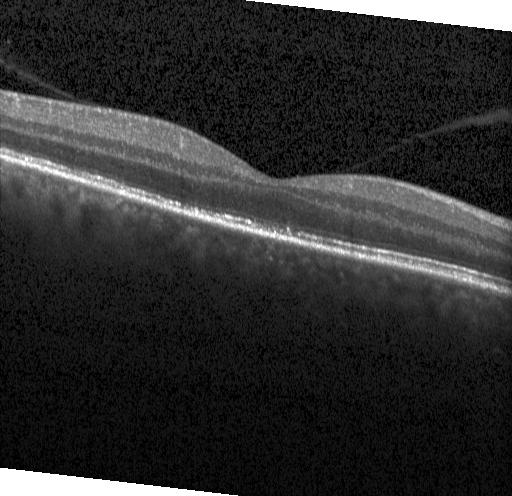
Diagnosis: no evidence of choroidal neovascularization, diabetic macular edema, or drusen.